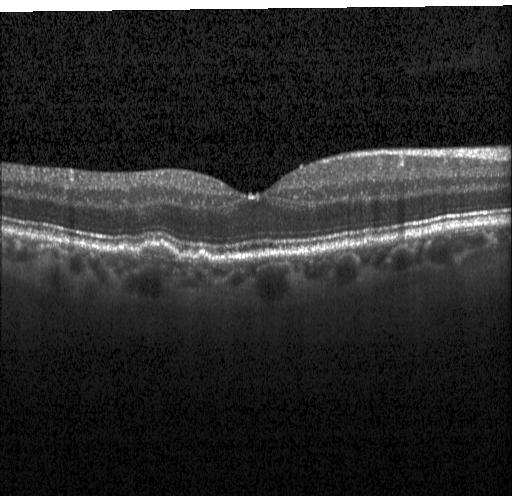
Retinal OCT cross-section showing multiple drusen.